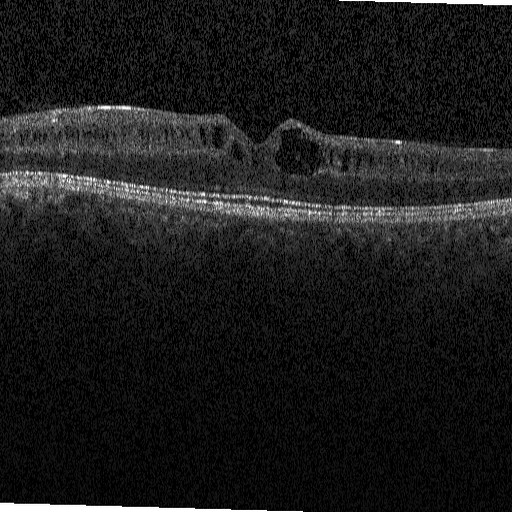

Retinal OCT cross-section. Spectral-domain optical coherence tomography. Horizontal scan through the fovea — OCT finding: DME.